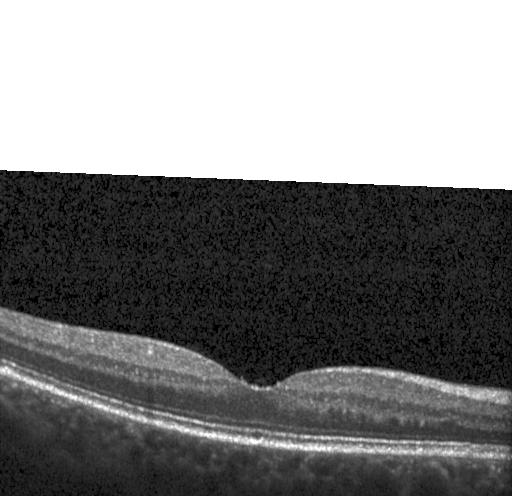 OCT line scan. Diagnosis: no CNV, DME, or drusen.